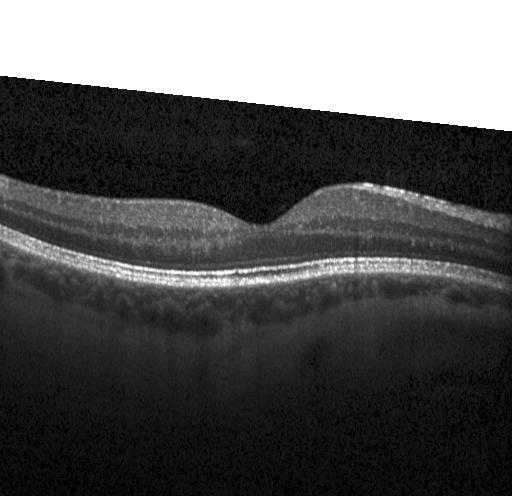
No evidence of CNV, DME, or drusen.